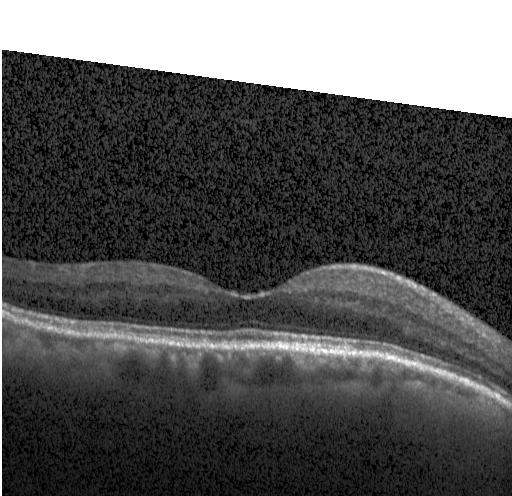
Finding: no evidence of choroidal neovascularization, diabetic macular edema, or drusen.